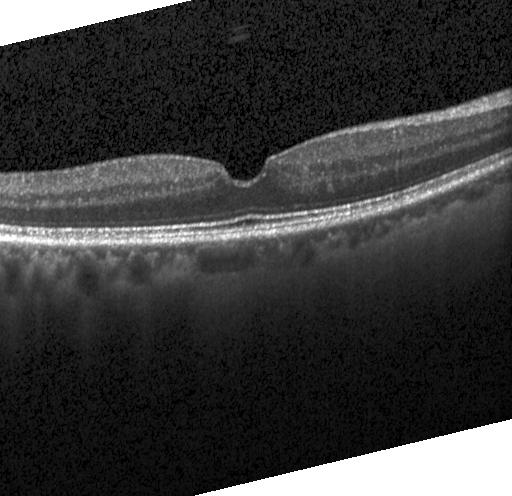
Finding: no evidence of choroidal neovascularization, diabetic macular edema, or drusen.